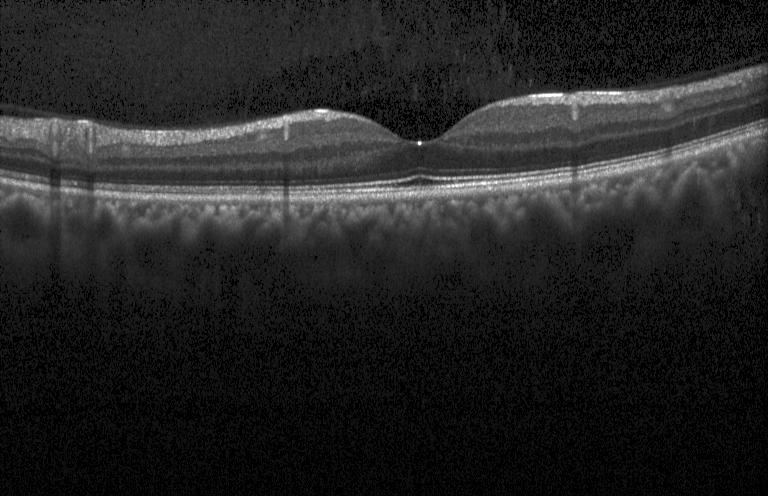

Heidelberg Spectralis OCT system · spectral-domain OCT · macular scan · optical coherence tomography B-scan — Diagnosis: no evidence of choroidal neovascularization, diabetic macular edema, or drusen.